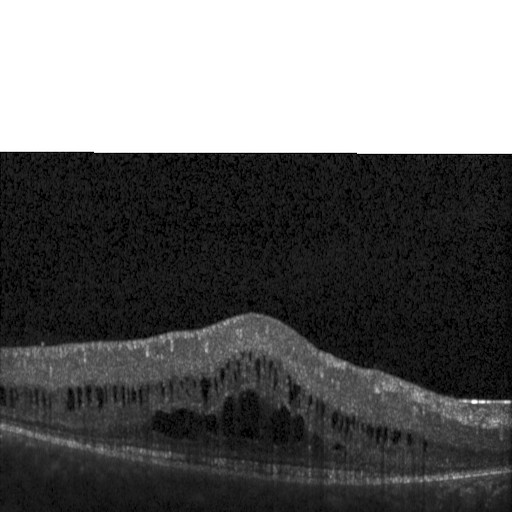
Optical coherence tomography B-scan. The scan shows DME.